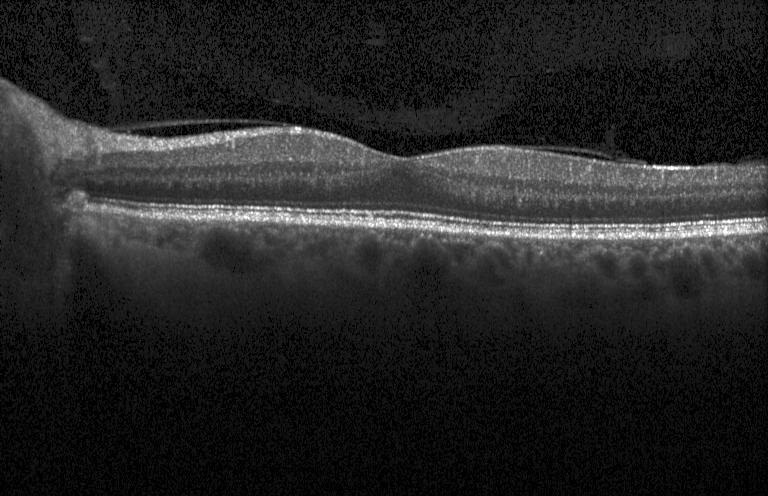

Optical coherence tomography B-scan, Heidelberg Spectralis, through the macula.
Dx: no choroidal neovascularization, no diabetic macular edema, and no drusen.